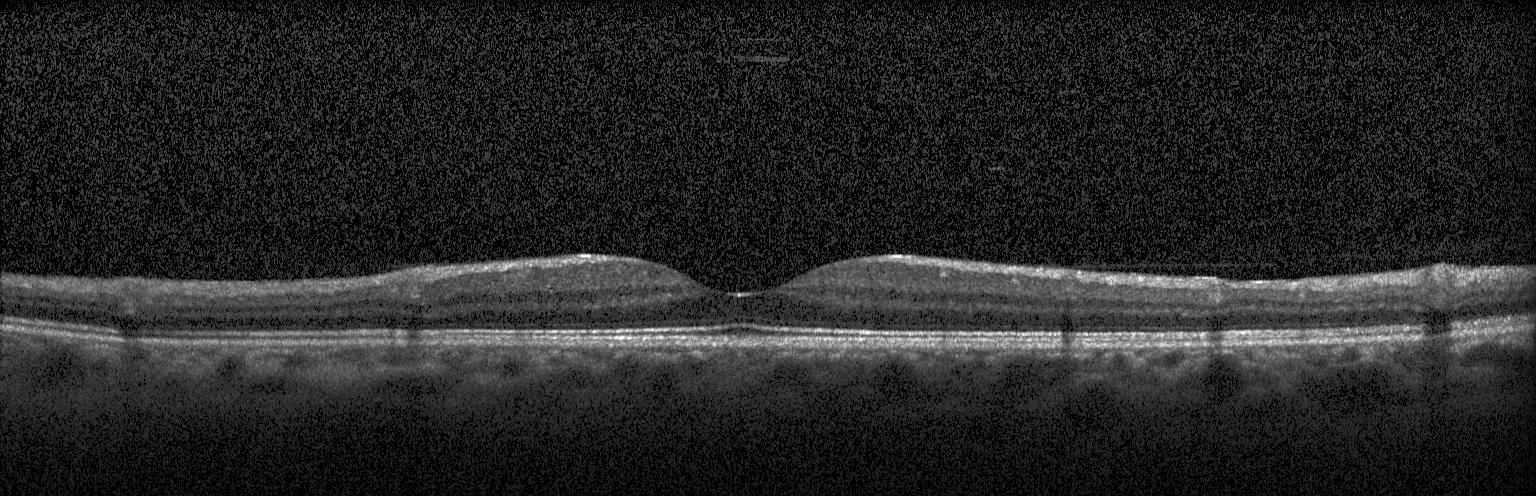 Heidelberg Spectralis OCT system, optical coherence tomography scan — Neither choroidal neovascularization, diabetic macular edema, nor drusen.